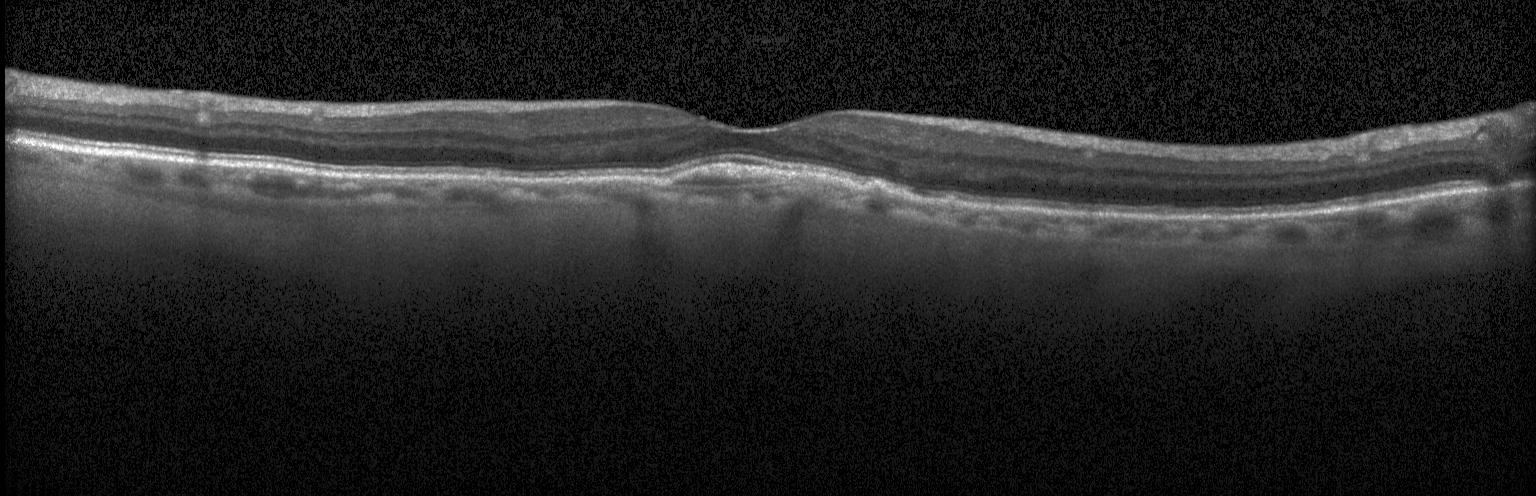 Retinal OCT cross-section showing a choroidal neovascular membrane.